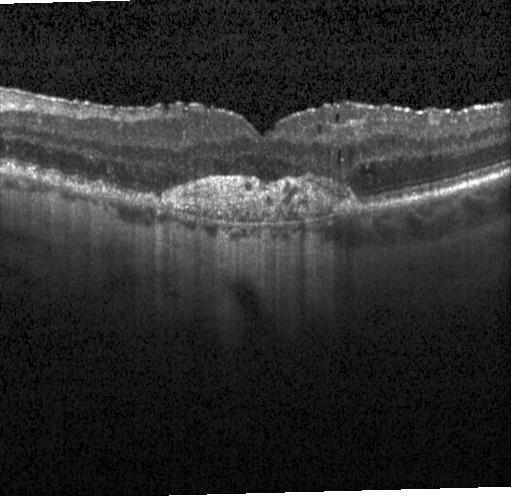 Heidelberg Spectralis · retinal OCT B-scan · horizontal scan through the fovea
Diagnosis: a choroidal neovascular membrane.